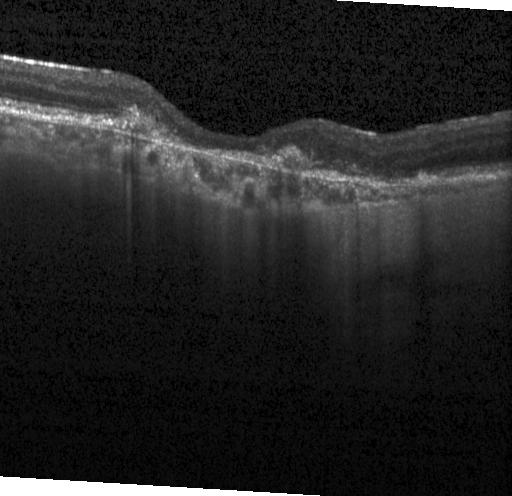

Optical coherence tomography scan
Assessment: choroidal neovascularization.